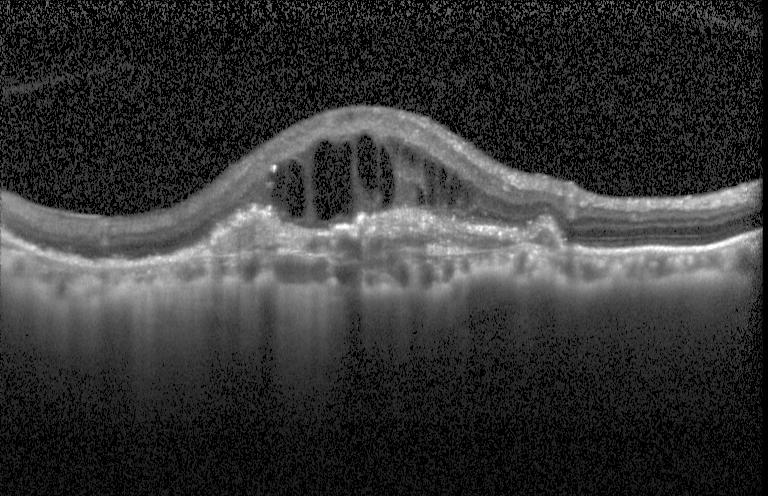
Acquired on a Heidelberg Spectralis · OCT B-scan — Macular OCT: a choroidal neovascular membrane.